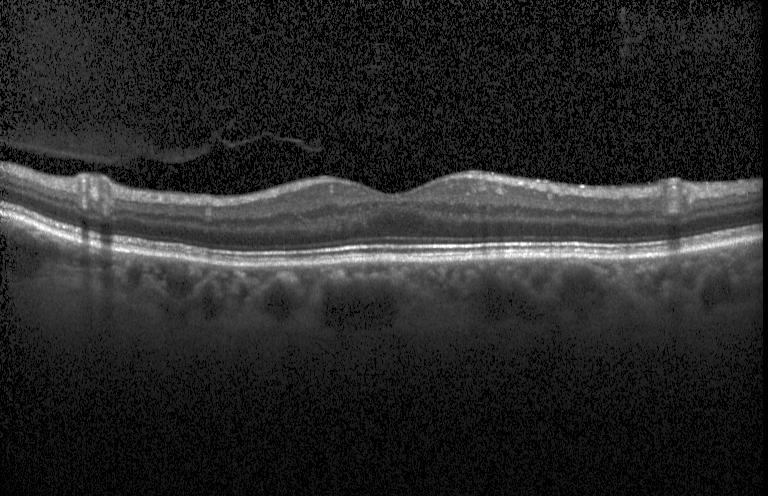

OCT line scan. Spectral-domain OCT. Centered on the fovea. Instrument: Heidelberg Spectralis
Diagnosis: no CNV, no DME, and no drusen.